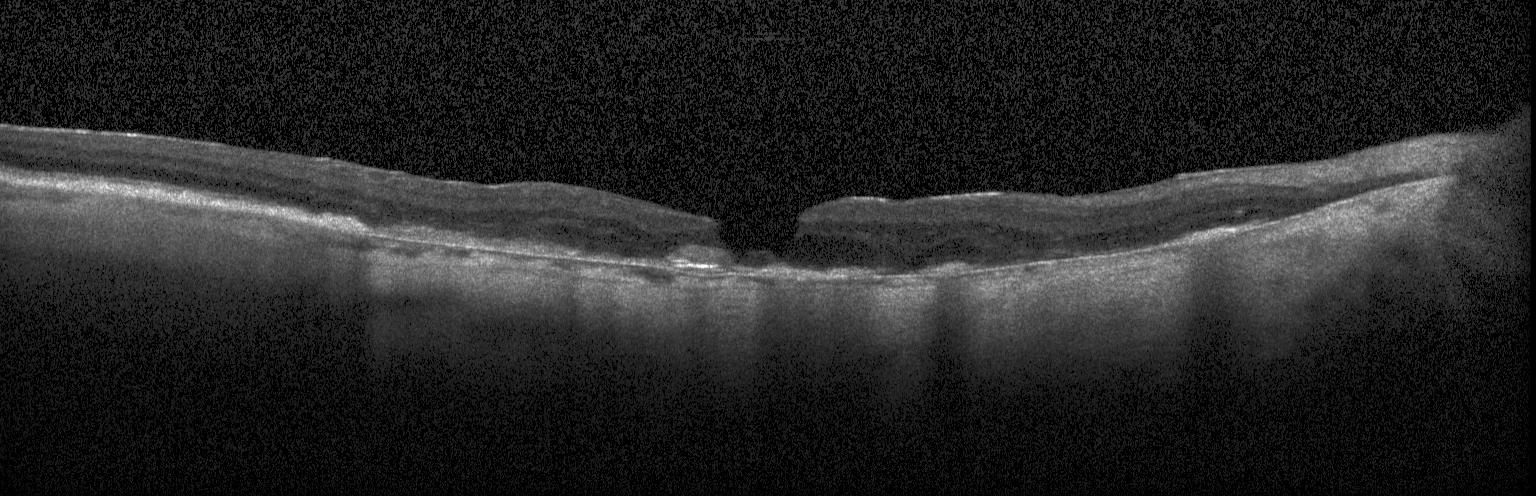
Horizontal scan through the fovea, spectral-domain optical coherence tomography, optical coherence tomography B-scan
This B-scan demonstrates choroidal neovascularization (CNV).